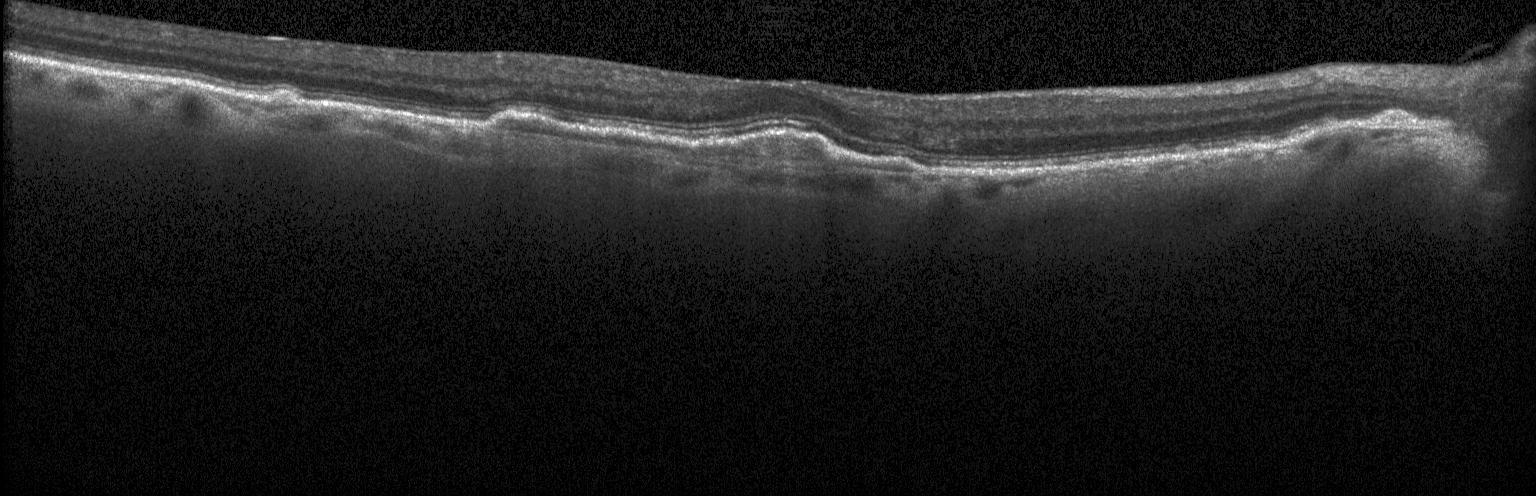 Retinal OCT B-scan; SD-OCT; macular scan. The scan shows choroidal neovascularization.